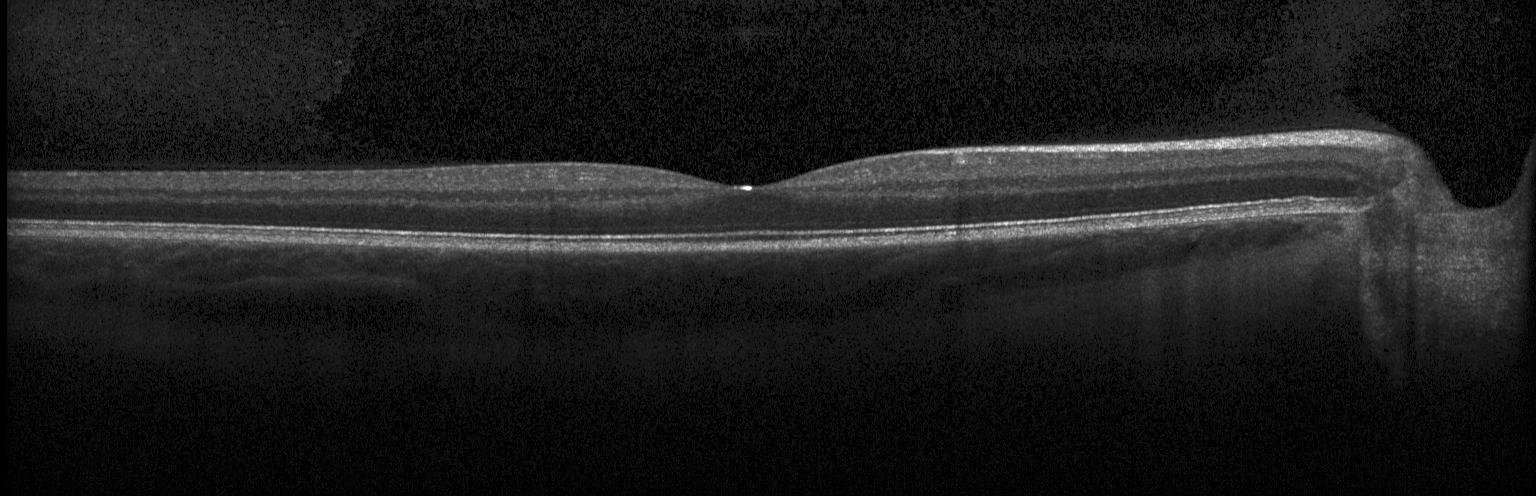

SD-OCT, instrument: Heidelberg Spectralis, macular scan, optical coherence tomography B-scan
Diagnosis: no evidence of CNV, DME, or drusen.